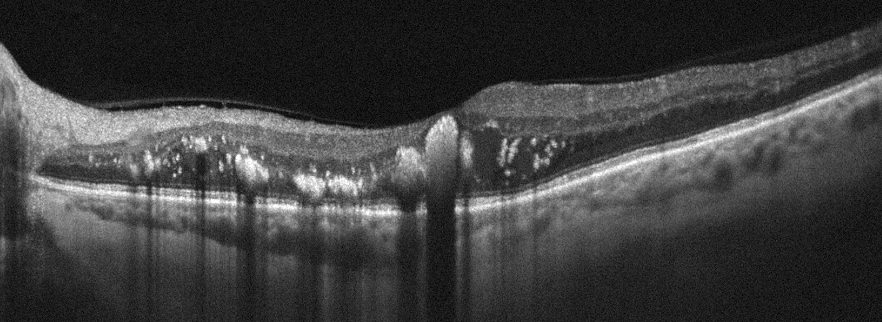

OCT line scan. Finding: diabetic macular edema.